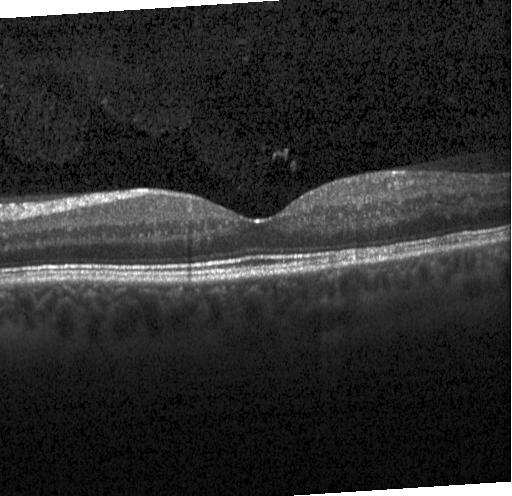

OCT finding: no evidence of choroidal neovascularization, diabetic macular edema, or drusen.